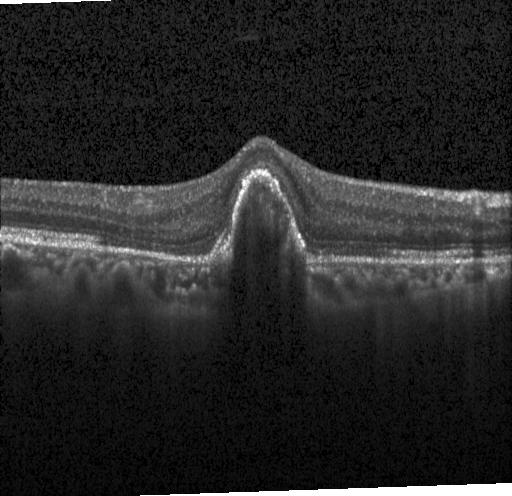
Optical coherence tomography scan · horizontal scan through the fovea · spectral-domain optical coherence tomography · Heidelberg Spectralis OCT system.
Diagnosis: a choroidal neovascular membrane.